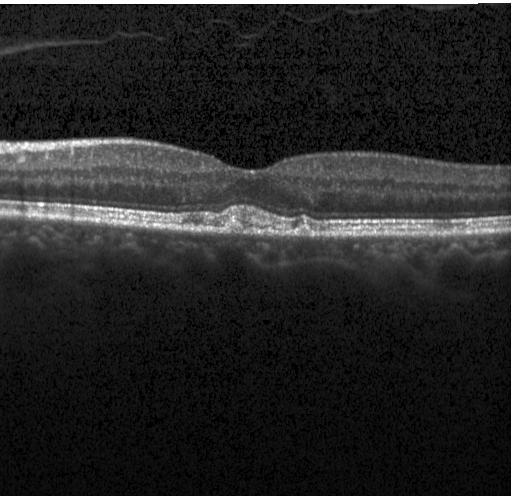
OCT B-scan showing sub-RPE drusenoid deposits.